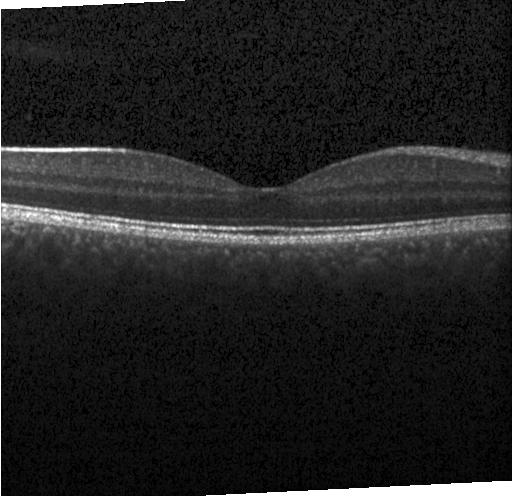 Impression: no choroidal neovascularization, no diabetic macular edema, and no drusen.